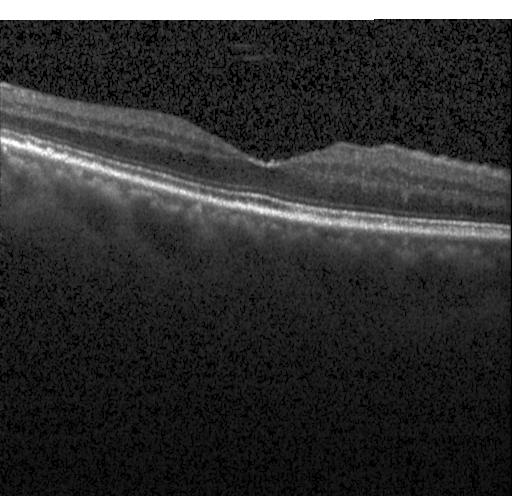

Retinal OCT B-scan, SD-OCT — No evidence of choroidal neovascularization, diabetic macular edema, or drusen.